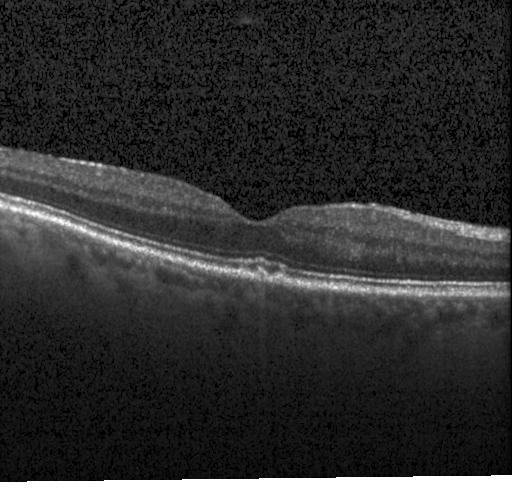

Spectral-domain optical coherence tomography, OCT line scan, macular scan. Impression: drusen.